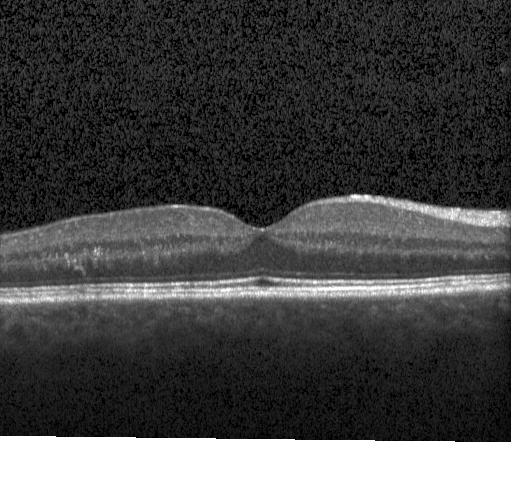 Assessment: no evidence of CNV, DME, or drusen.